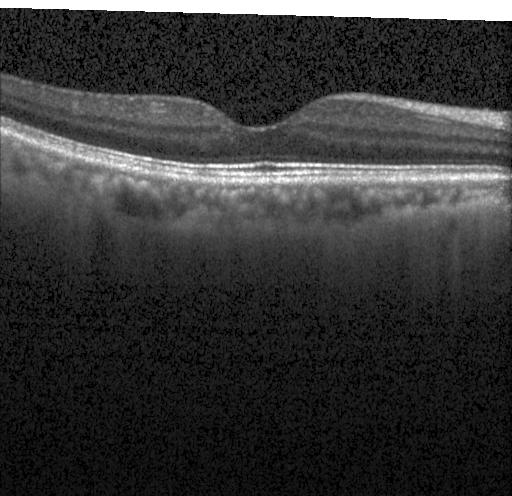
Retinal OCT cross-section · macular scan — Finding: no evidence of choroidal neovascularization, diabetic macular edema, or drusen.